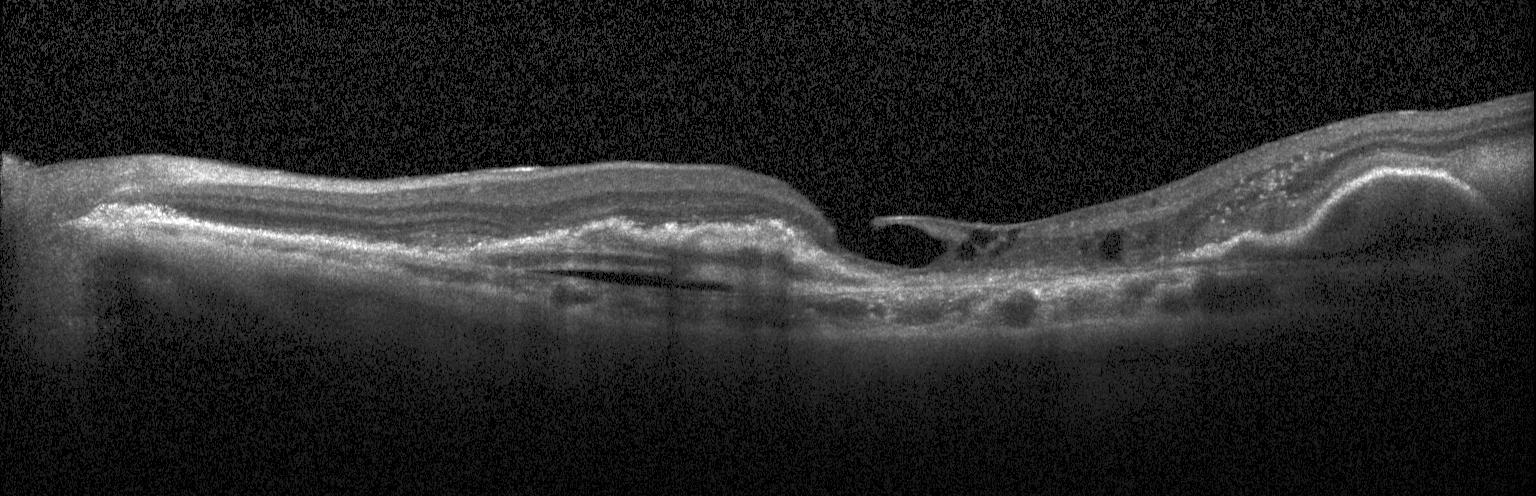
Macular OCT: a choroidal neovascular membrane.